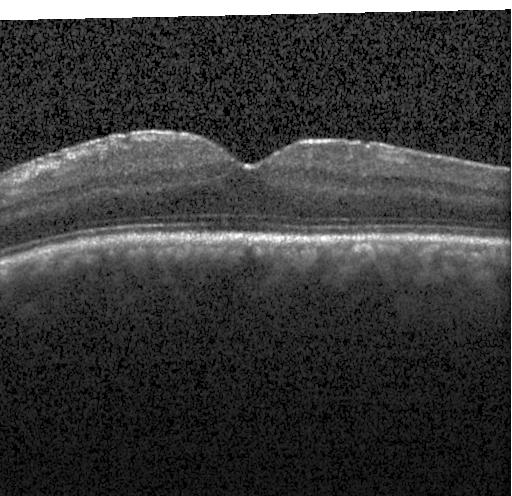

Optical coherence tomography scan; spectral-domain optical coherence tomography.
Impression: neither CNV, DME, nor drusen.